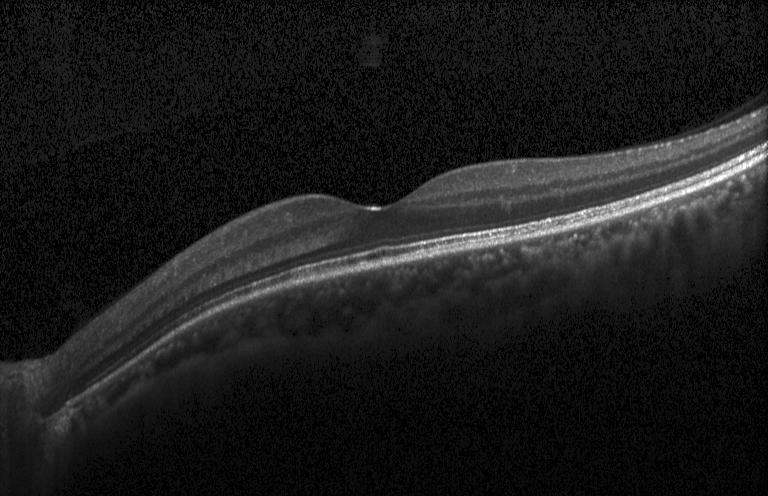 Horizontal scan through the fovea, retinal OCT B-scan, instrument: Heidelberg Spectralis.
Diagnosis: no CNV, no DME, and no drusen.